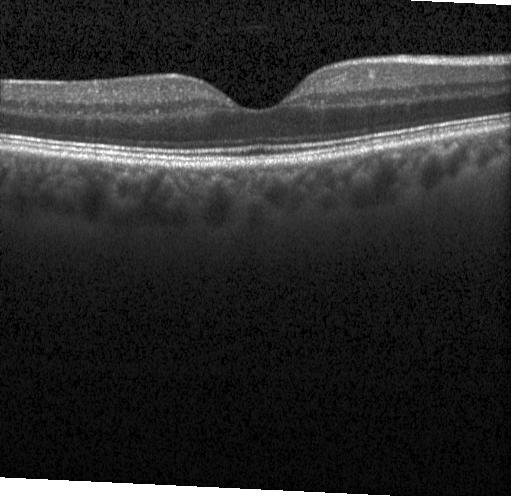 OCT B-scan. Heidelberg Spectralis
No choroidal neovascularization, no diabetic macular edema, and no drusen.